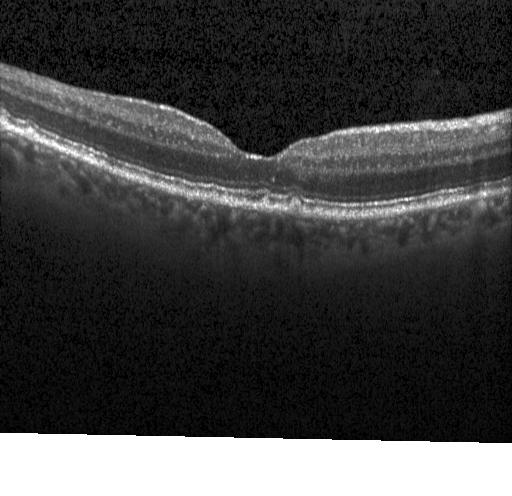 Retinal OCT B-scan — Assessment: drusen.